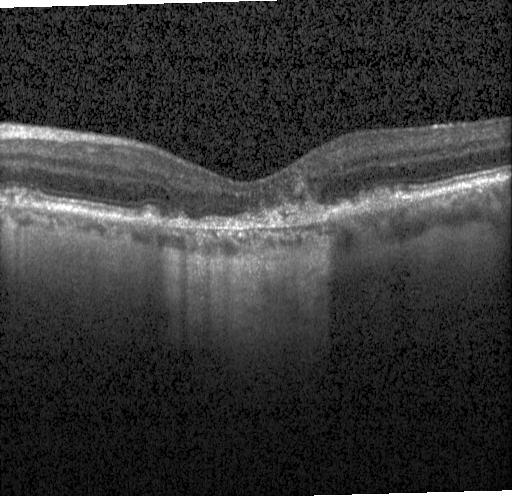 Diagnosis: a choroidal neovascular membrane.